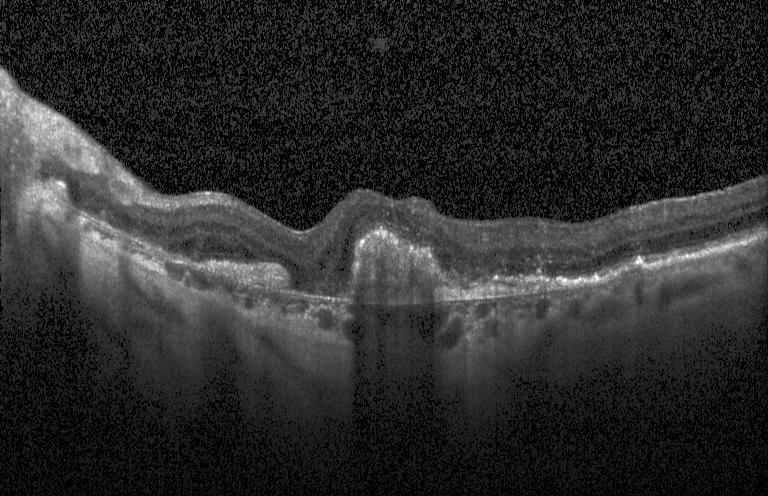

Heidelberg Spectralis · spectral-domain OCT · OCT B-scan · fovea-centered. Macular OCT: a choroidal neovascular membrane.